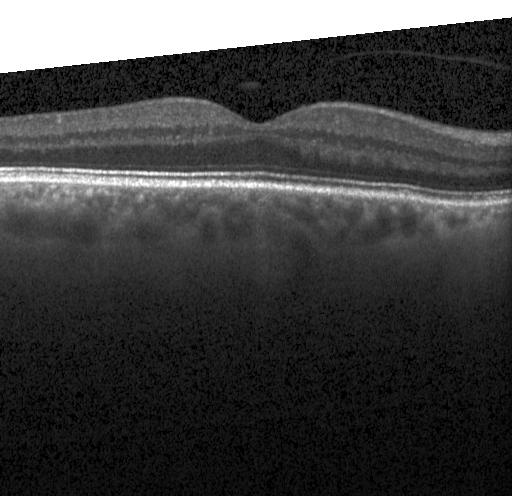
Optical coherence tomography scan. Impression: no evidence of choroidal neovascularization, diabetic macular edema, or drusen.